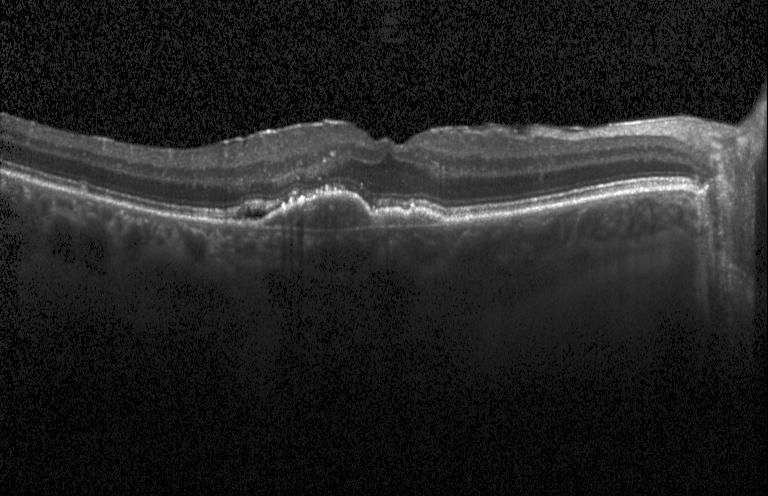

Heidelberg Spectralis OCT system · optical coherence tomography B-scan — Diagnosis: a choroidal neovascular membrane.